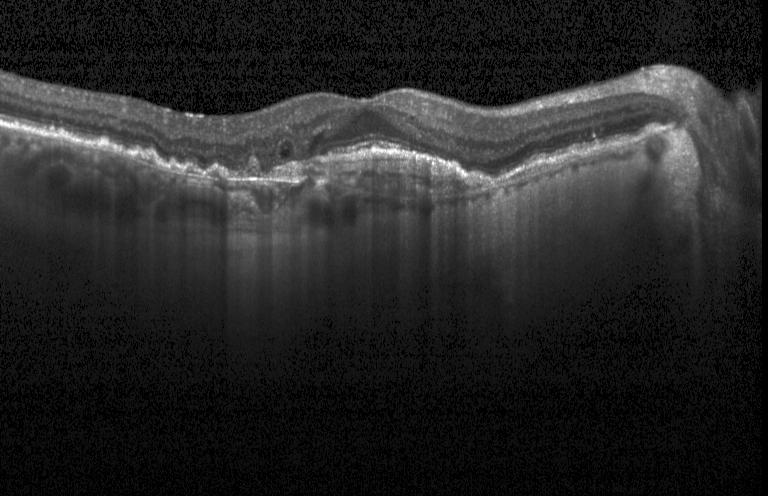
Optical coherence tomography B-scan. Fovea-centered. SD-OCT
Impression: CNV.